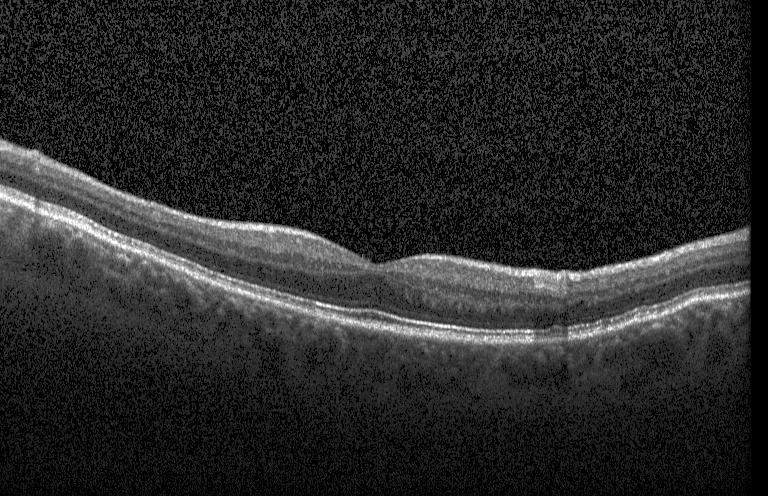
Heidelberg Spectralis. OCT B-scan. Assessment: no choroidal neovascularization, no diabetic macular edema, and no drusen.